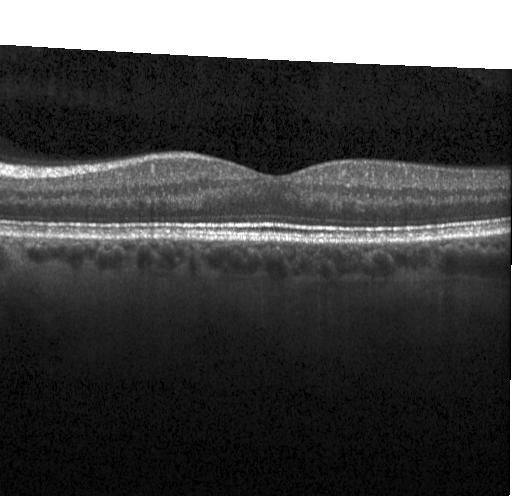

Instrument: Heidelberg Spectralis; OCT B-scan; SD-OCT — Impression: no choroidal neovascularization, diabetic macular edema, or drusen.